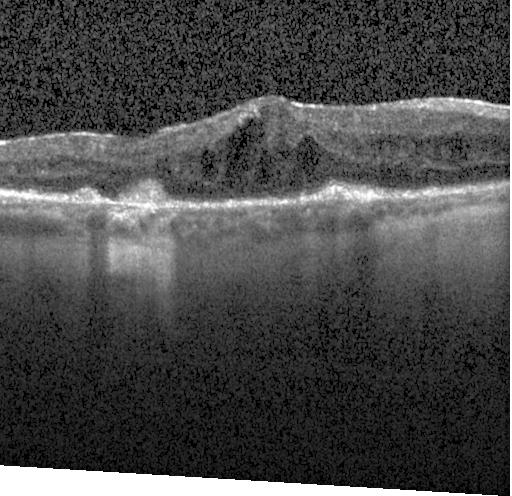 Heidelberg Spectralis OCT system · retinal OCT B-scan — The scan shows a choroidal neovascular membrane.